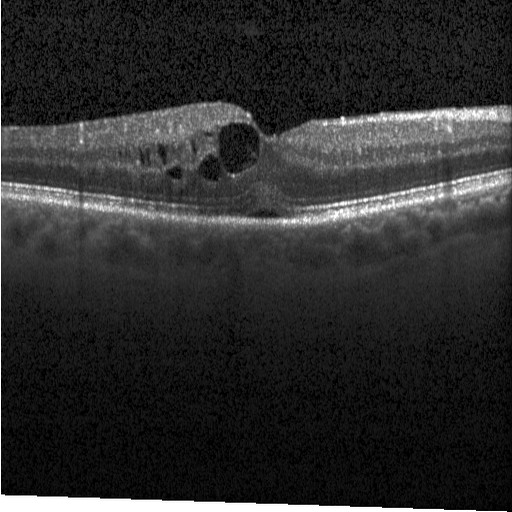

Spectral-domain optical coherence tomography · OCT B-scan.
OCT finding: diabetic macular edema.